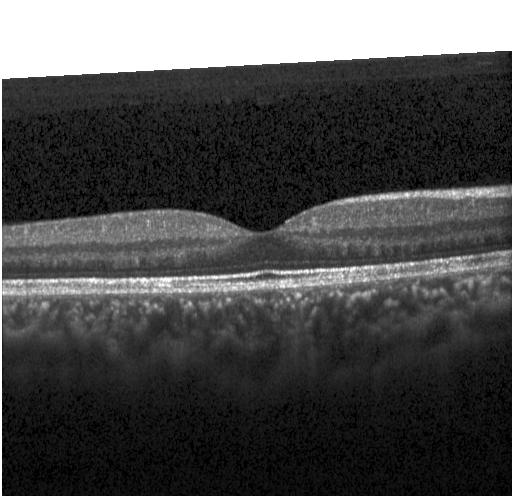 SD-OCT; macular scan; acquired on a Heidelberg Spectralis; retinal OCT cross-section.
Diagnosis: no choroidal neovascularization, no diabetic macular edema, and no drusen.